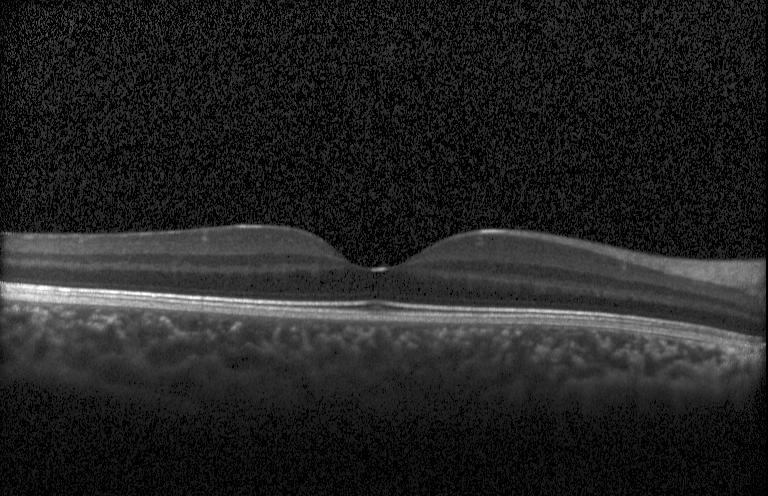

Centered on the fovea · OCT line scan · instrument: Heidelberg Spectralis
Finding: no CNV, no DME, and no drusen.